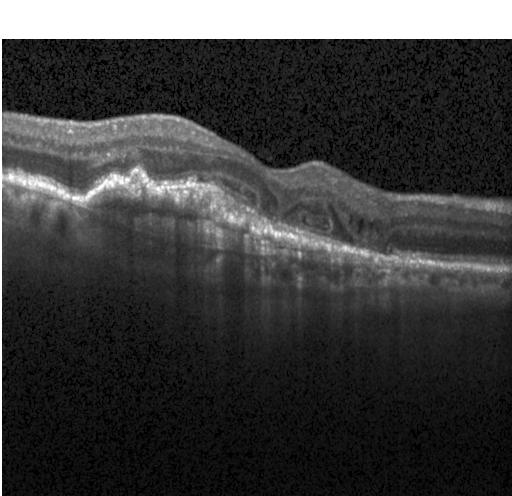 The scan shows CNV.